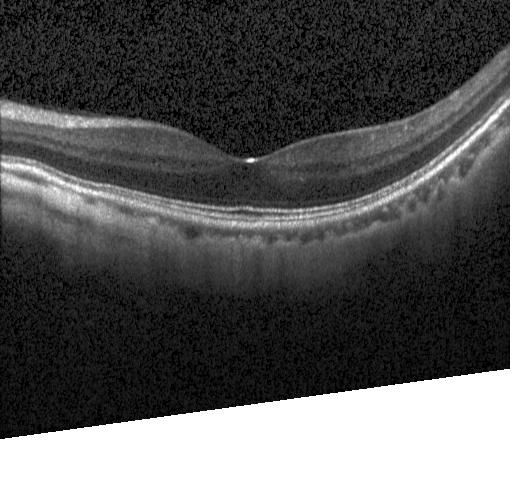 Macular OCT demonstrating no evidence of choroidal neovascularization, diabetic macular edema, or drusen.